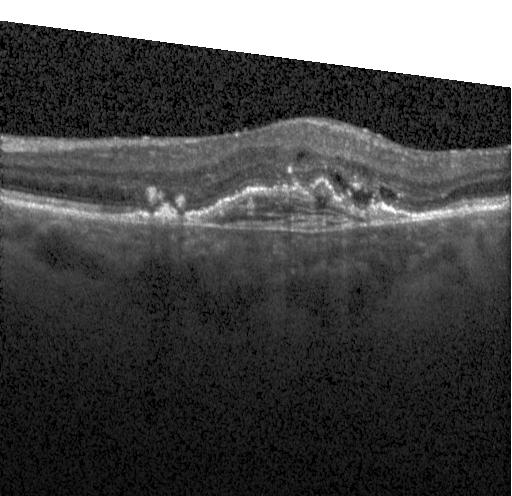

Spectral-domain OCT · Heidelberg Spectralis OCT system · retinal OCT B-scan · centered on the fovea — Diagnosis: CNV.